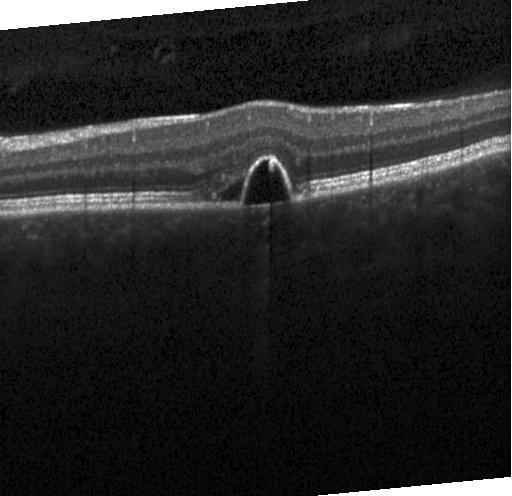
Assessment: a choroidal neovascular membrane.